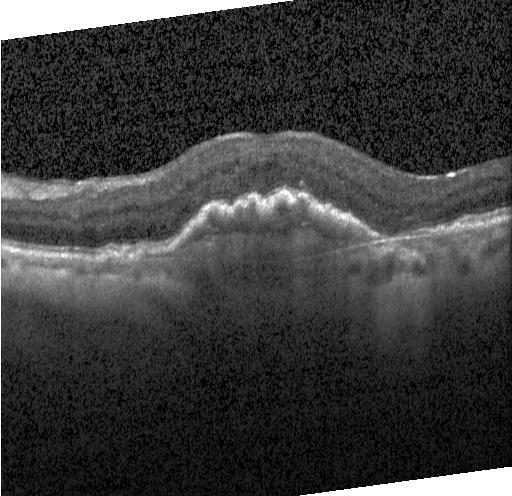

The scan shows a choroidal neovascular membrane.